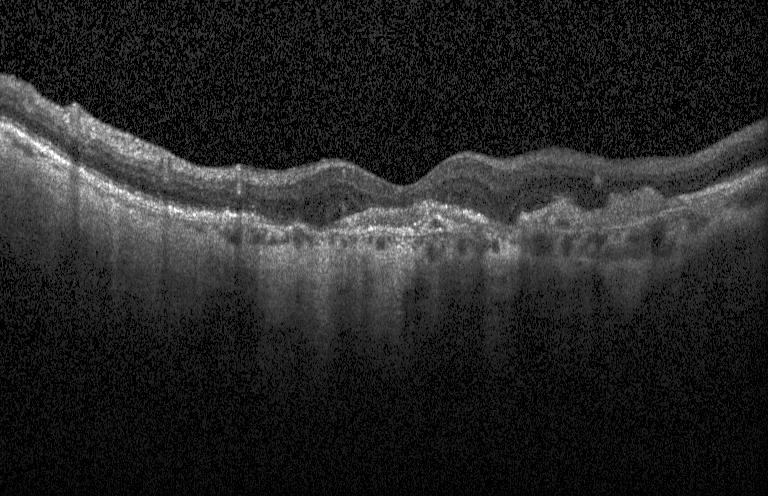 Dx: a choroidal neovascular membrane.